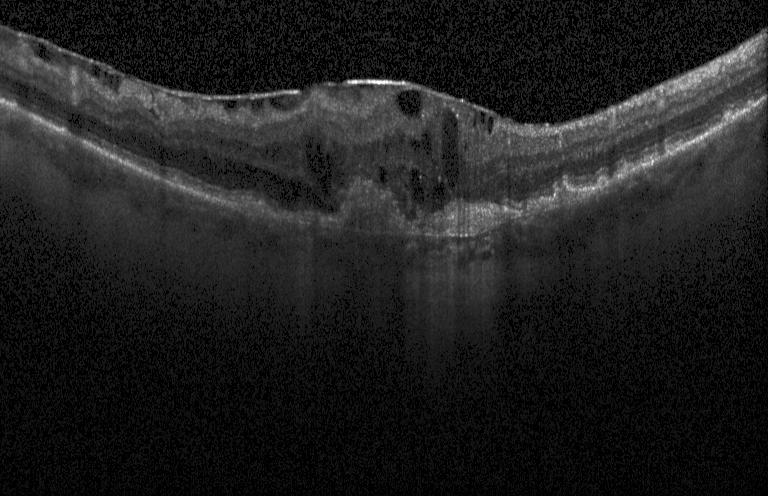
Retinal OCT cross-section. The scan shows choroidal neovascularization (CNV).